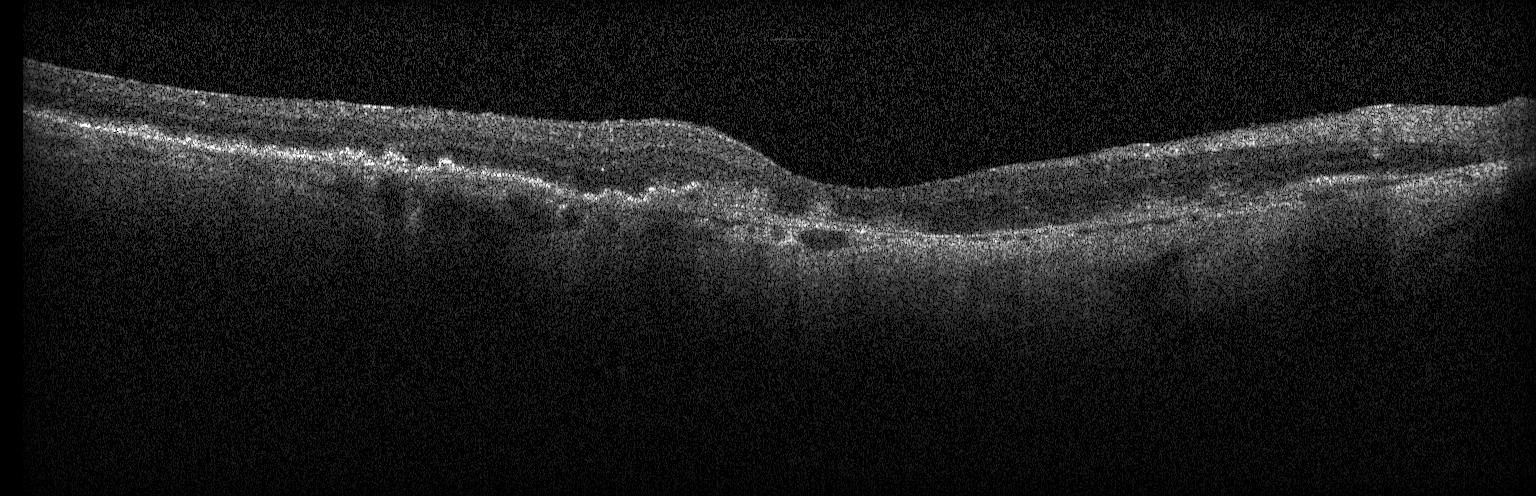

Retinal OCT B-scan — Finding: choroidal neovascularization.